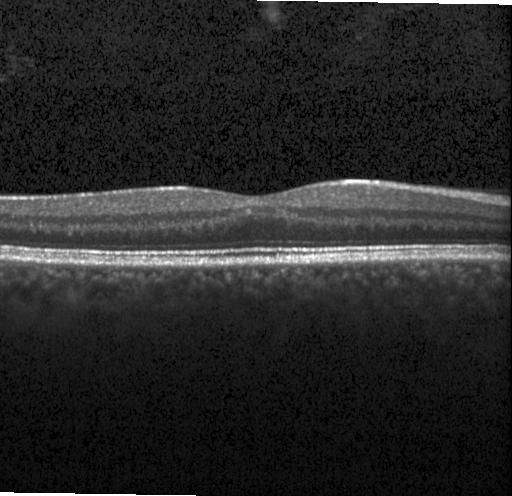
Diagnosis: neither choroidal neovascularization, diabetic macular edema, nor drusen.